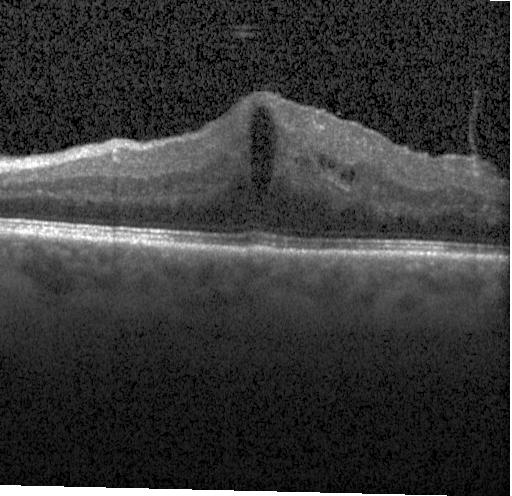
OCT line scan. Impression: diabetic macular edema.